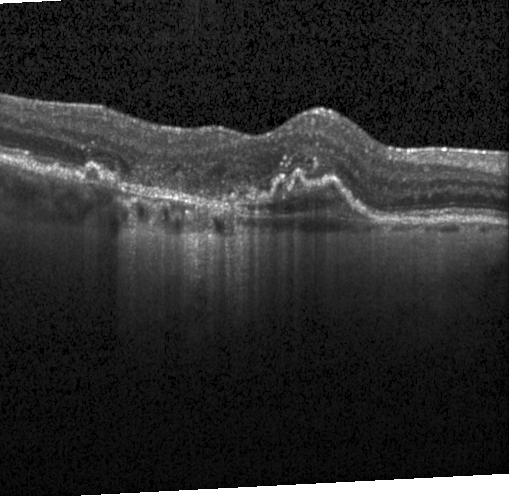 Retinal OCT cross-section
This B-scan demonstrates CNV.